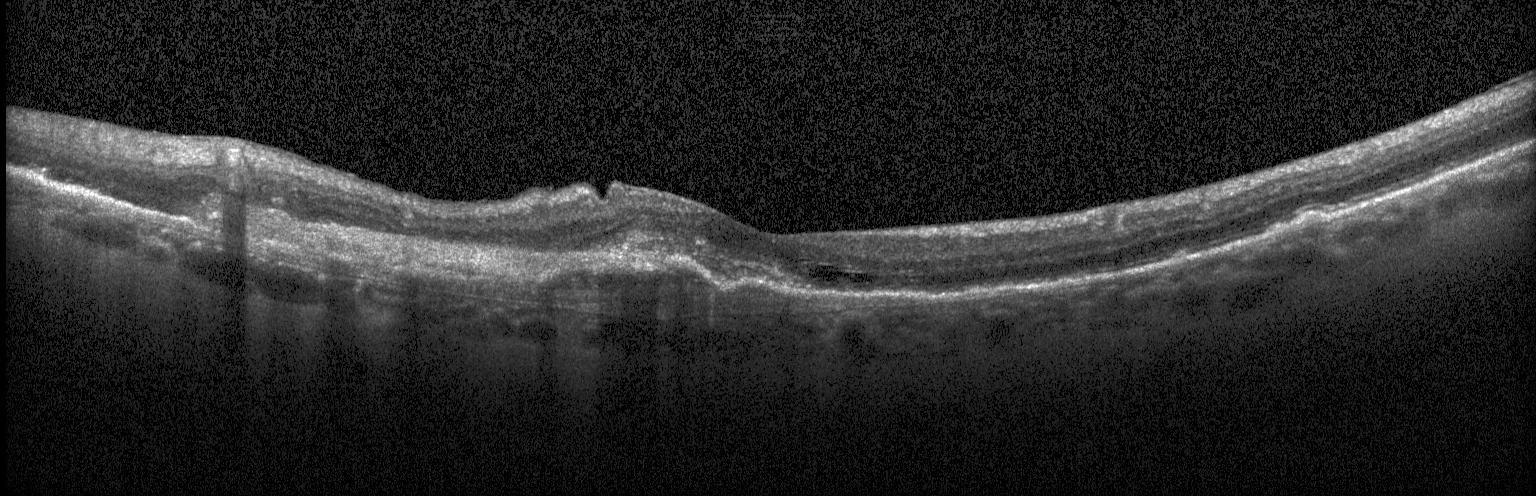 Finding: a choroidal neovascular membrane.